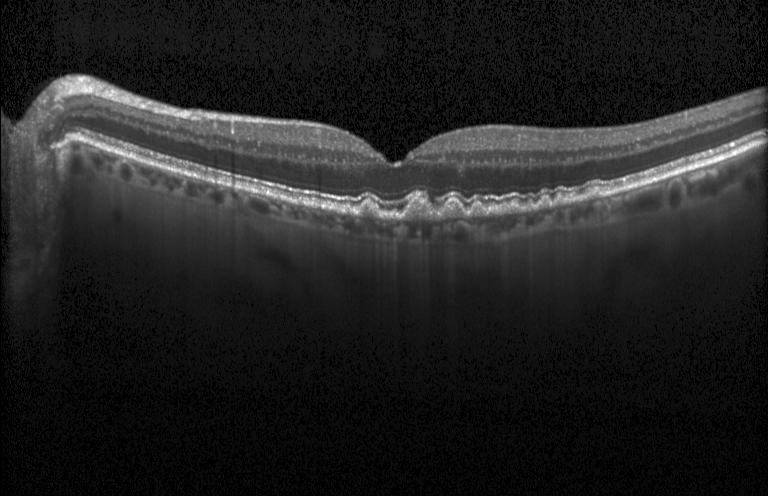

Macular OCT: drusen.